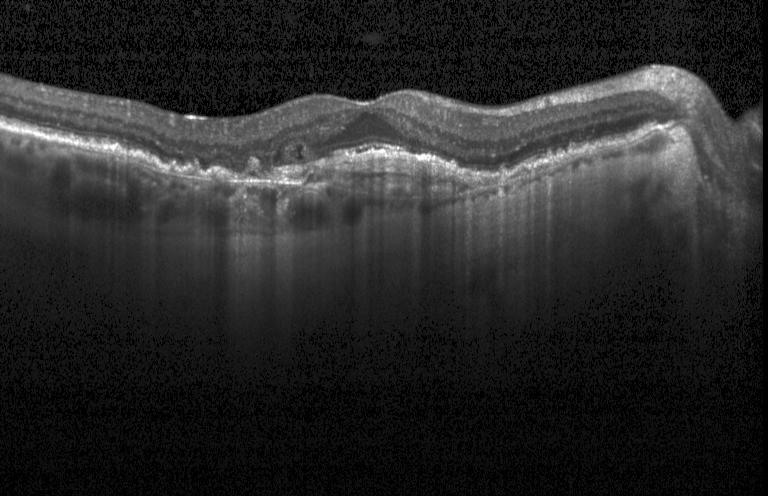

Retinal OCT cross-section showing choroidal neovascularization (CNV).